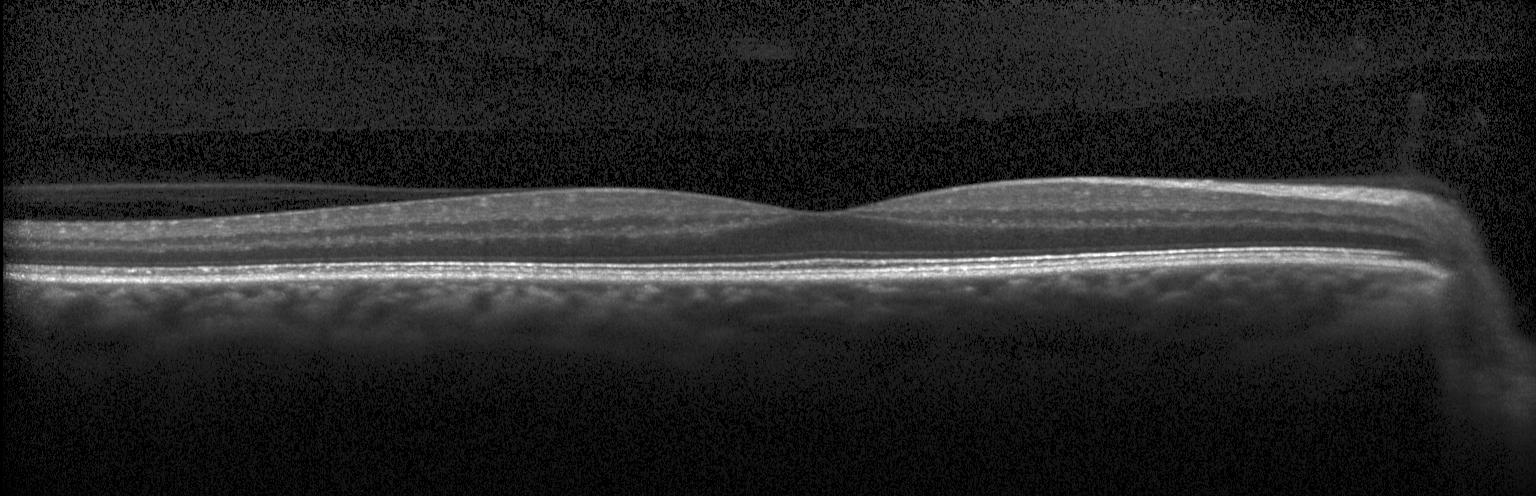

Acquired on a Heidelberg Spectralis; spectral-domain optical coherence tomography; OCT B-scan. Diagnosis: no evidence of choroidal neovascularization, diabetic macular edema, or drusen.